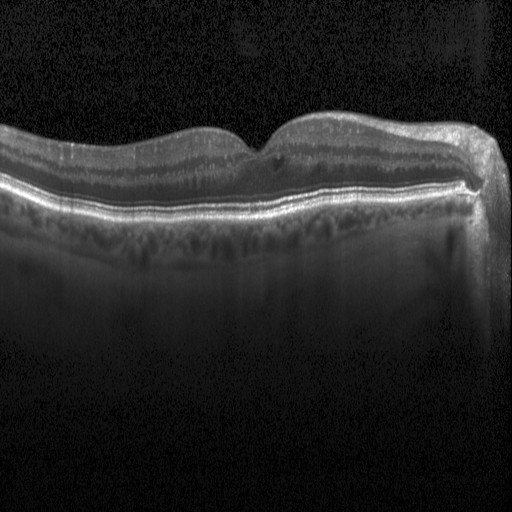

Macular OCT: diabetic macular edema (DME).